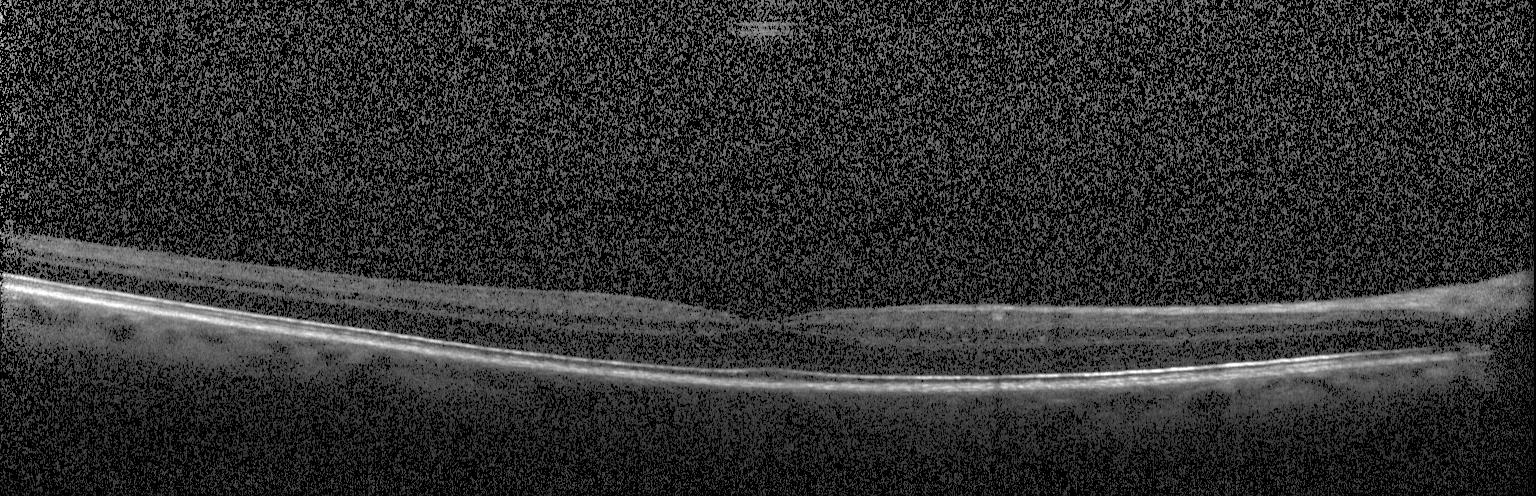
Retinal OCT cross-section showing neither choroidal neovascularization, diabetic macular edema, nor drusen.